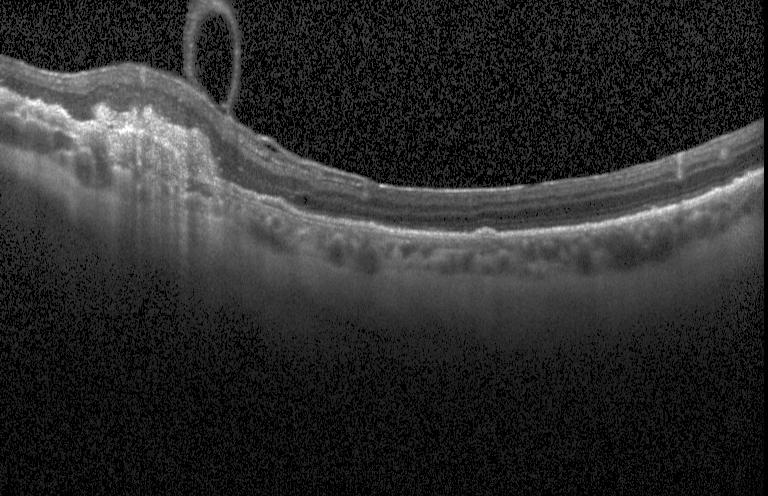
Diagnosis: choroidal neovascularization.